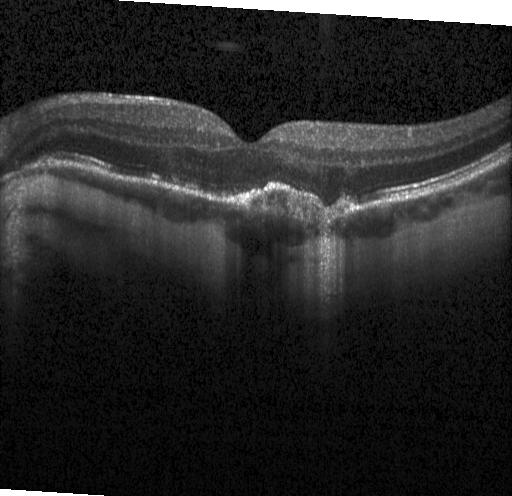

Spectral-domain OCT B-scan: choroidal neovascularization (CNV).